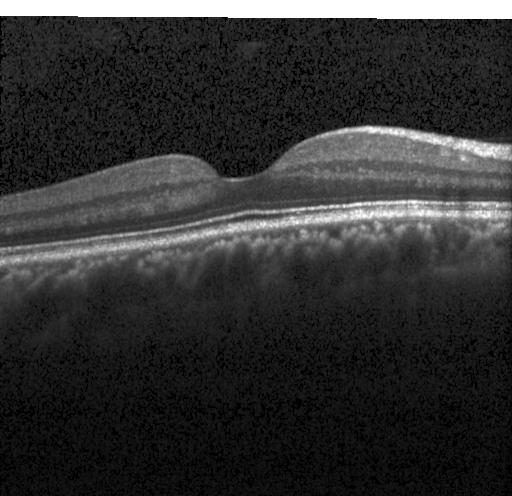 Retinal OCT cross-section showing no evidence of CNV, DME, or drusen.